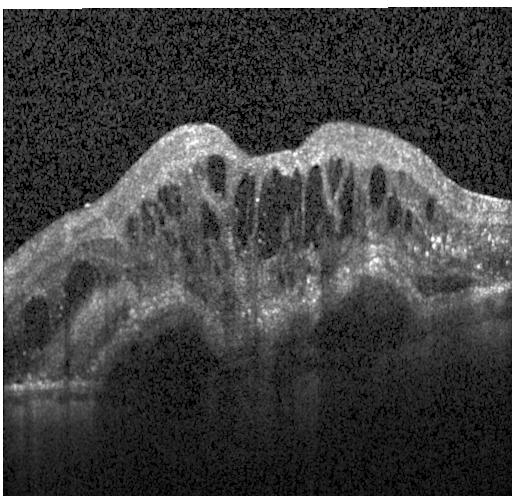
OCT B-scan. Through the macula. Instrument: Heidelberg Spectralis
The scan shows a choroidal neovascular membrane.